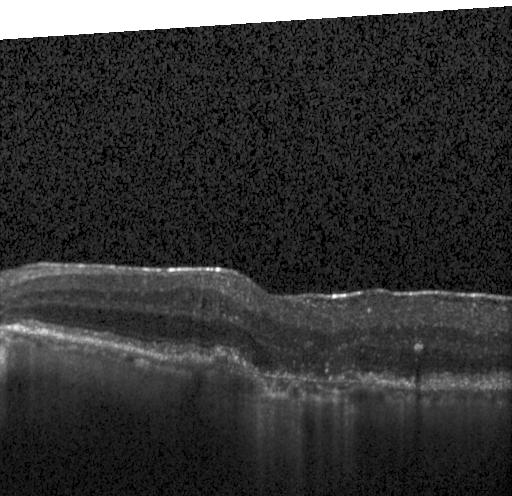

Macular OCT demonstrating choroidal neovascularization (CNV).